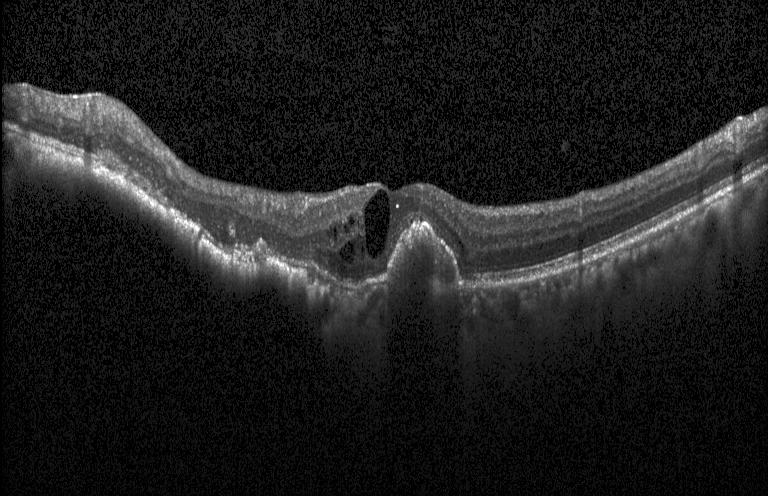

OCT B-scan; instrument: Heidelberg Spectralis
Choroidal neovascularization.